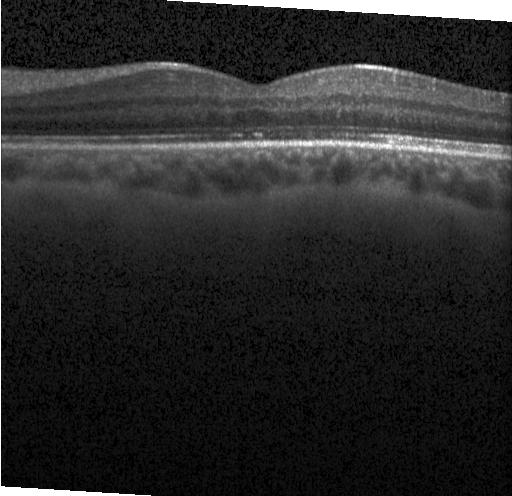

Dx: no choroidal neovascularization, no diabetic macular edema, and no drusen.